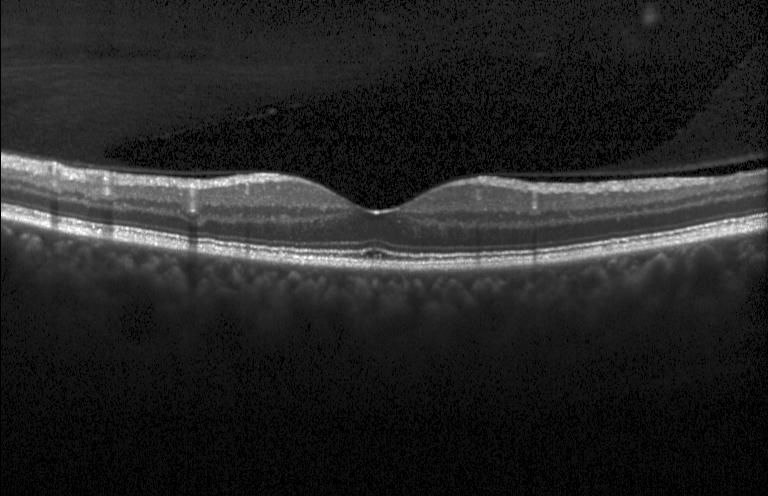

Dx: no choroidal neovascularization, no diabetic macular edema, and no drusen.